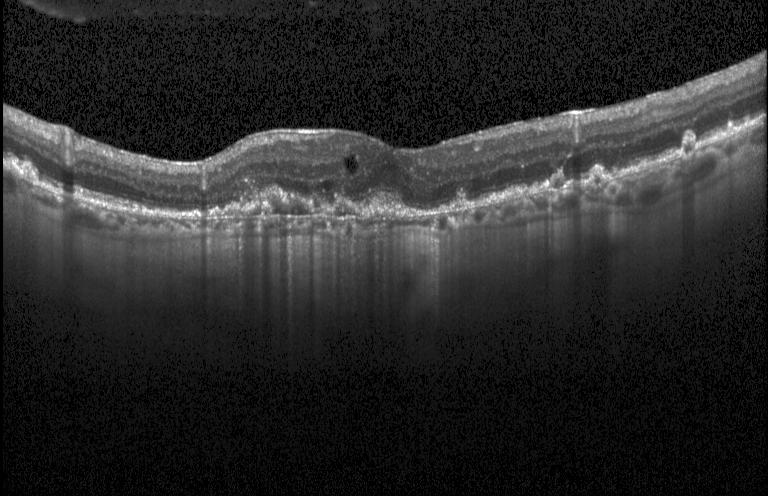 Instrument: Heidelberg Spectralis. Spectral-domain OCT. Horizontal scan through the fovea. OCT line scan. Diagnosis: a choroidal neovascular membrane.